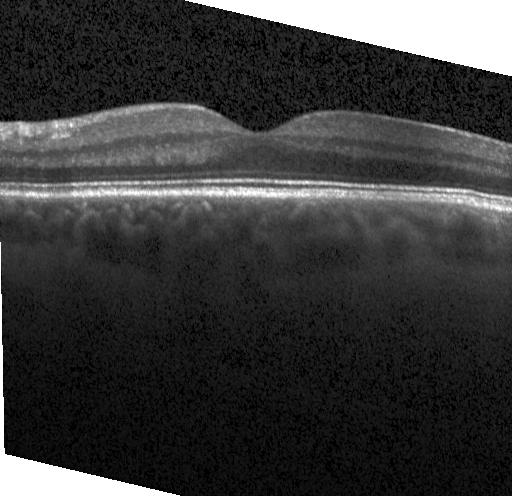
OCT scan showing no choroidal neovascularization, diabetic macular edema, or drusen.